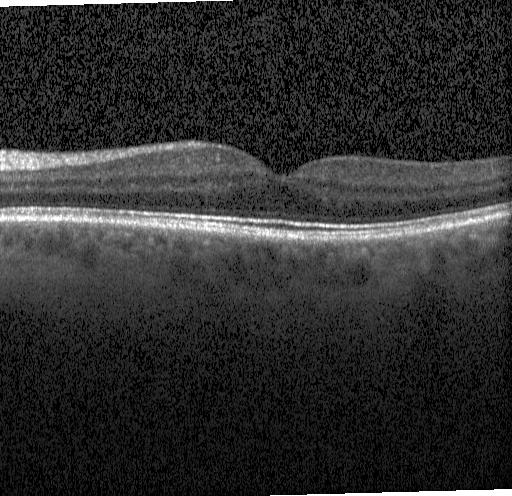

Optical coherence tomography B-scan.
Diagnosis: no CNV, no DME, and no drusen.